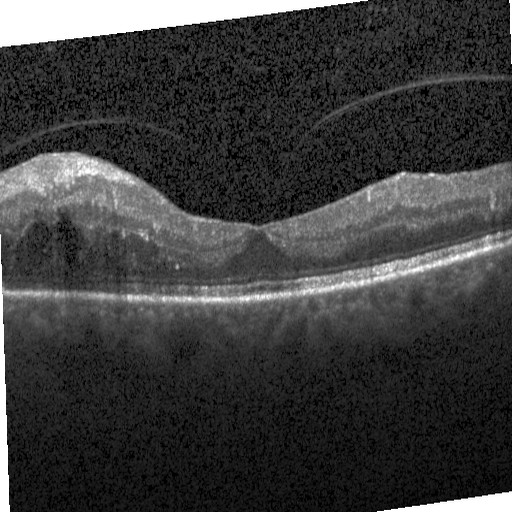 Optical coherence tomography scan. Heidelberg Spectralis OCT system — Diagnosis: DME.